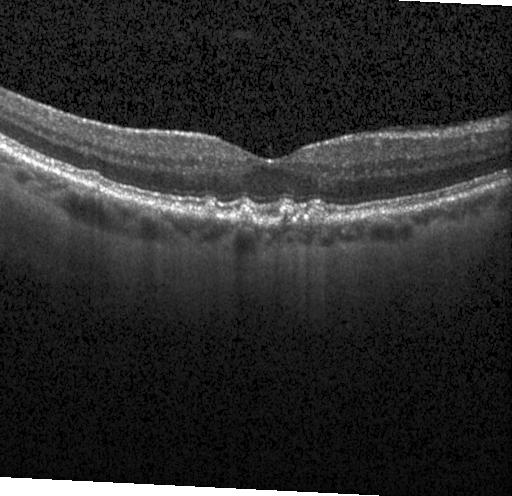
Optical coherence tomography scan, macular scan.
Sub-RPE drusenoid deposits.